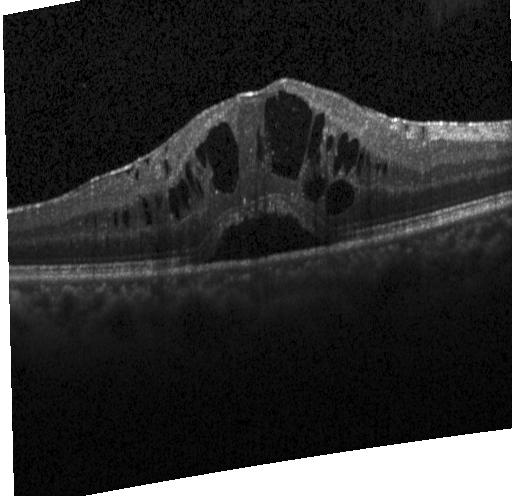 Acquired on a Heidelberg Spectralis · spectral-domain optical coherence tomography · horizontal scan through the fovea · optical coherence tomography B-scan. Impression: diabetic macular edema.